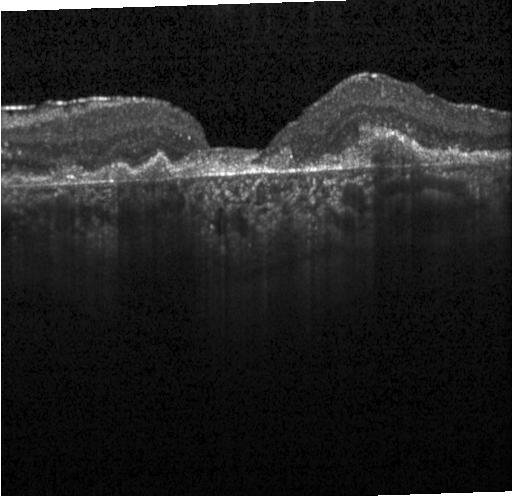
Spectral-domain OCT · Heidelberg Spectralis · OCT line scan.
A choroidal neovascular membrane.